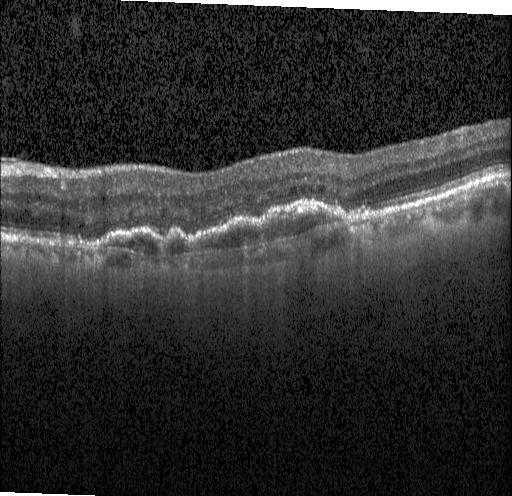
OCT B-scan showing CNV.